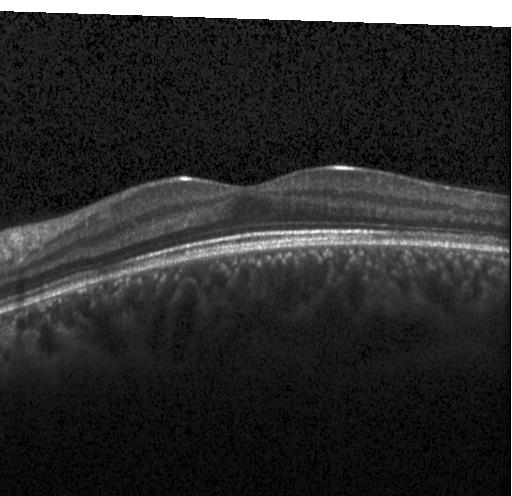
OCT B-scan, Heidelberg Spectralis, through the macula
This B-scan demonstrates no evidence of CNV, DME, or drusen.